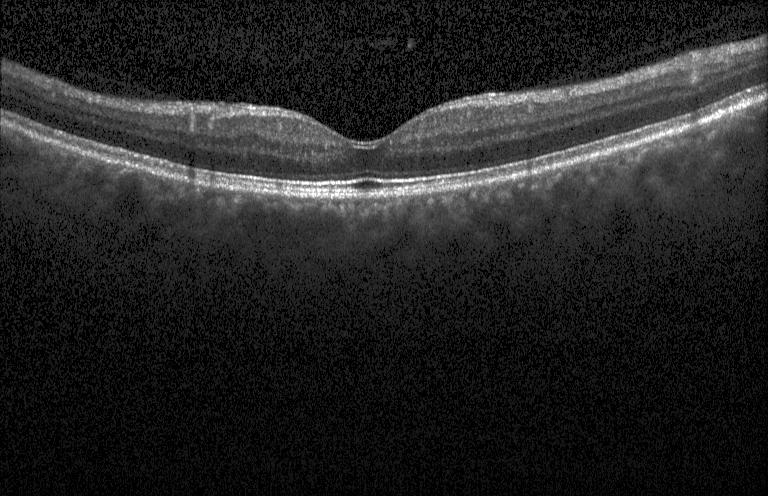
No choroidal neovascularization, no diabetic macular edema, and no drusen.